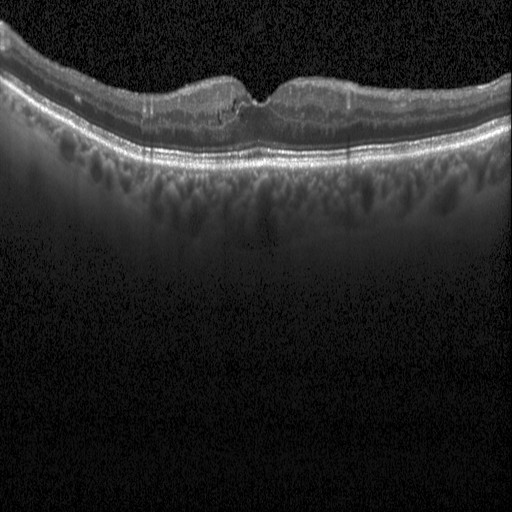 Acquired on a Heidelberg Spectralis · OCT B-scan
Diagnosis: DME.